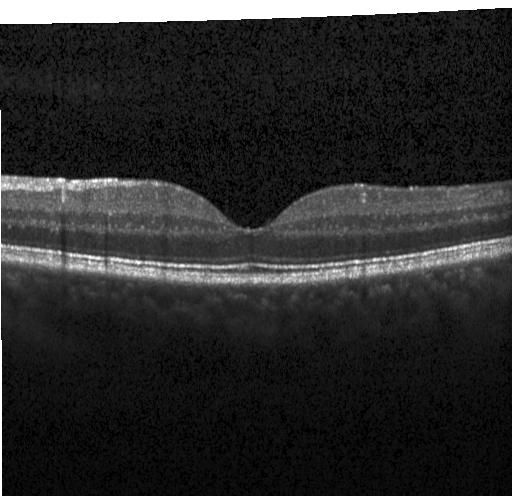
Optical coherence tomography scan — Dx: no choroidal neovascularization, diabetic macular edema, or drusen.